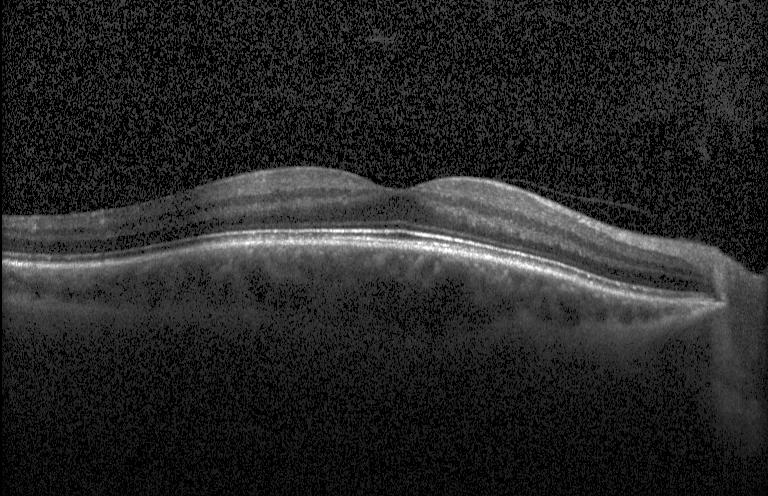

Retinal OCT B-scan — Diagnosis: no choroidal neovascularization, no diabetic macular edema, and no drusen.